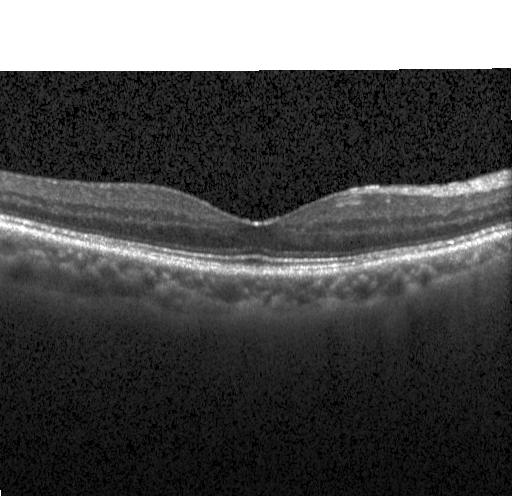

Macular scan. OCT line scan
Impression: no evidence of choroidal neovascularization, diabetic macular edema, or drusen.